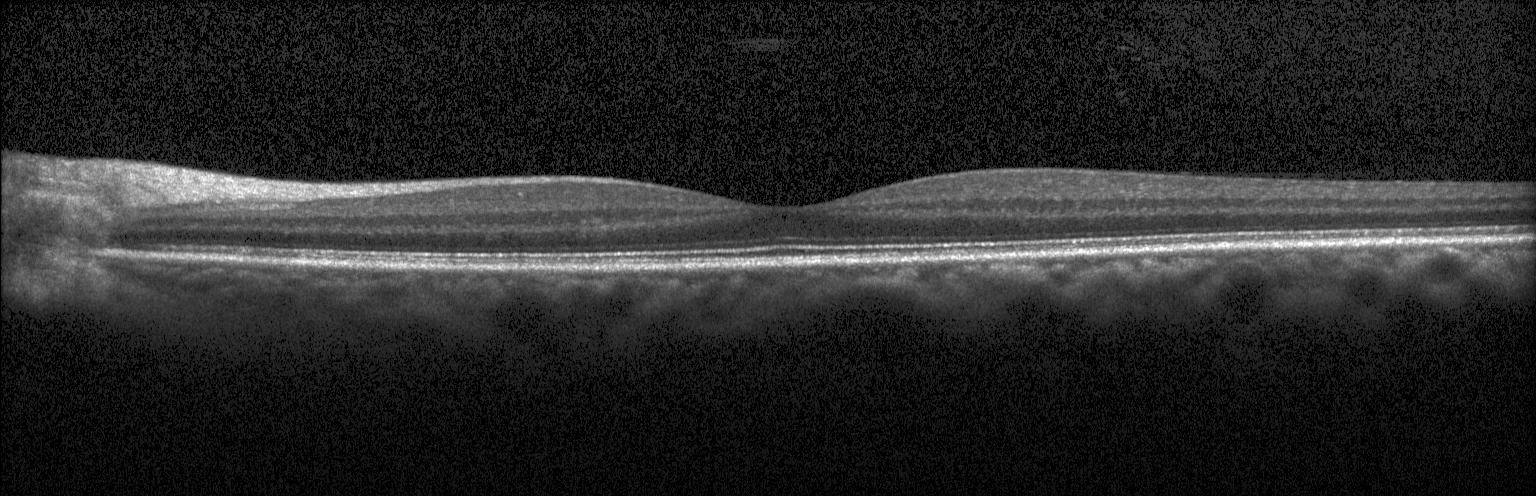
Spectral-domain OCT. Retinal OCT cross-section. No choroidal neovascularization, no diabetic macular edema, and no drusen.